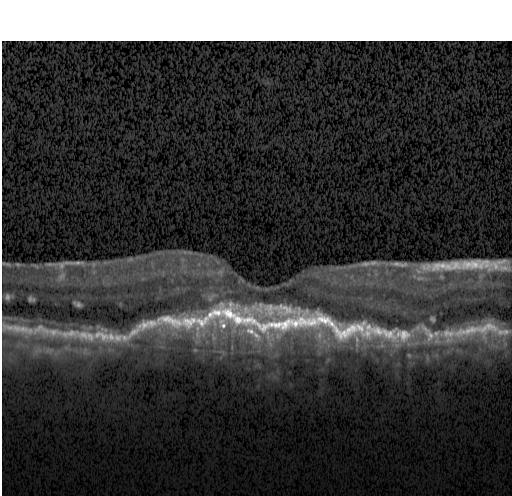 Finding: CNV.